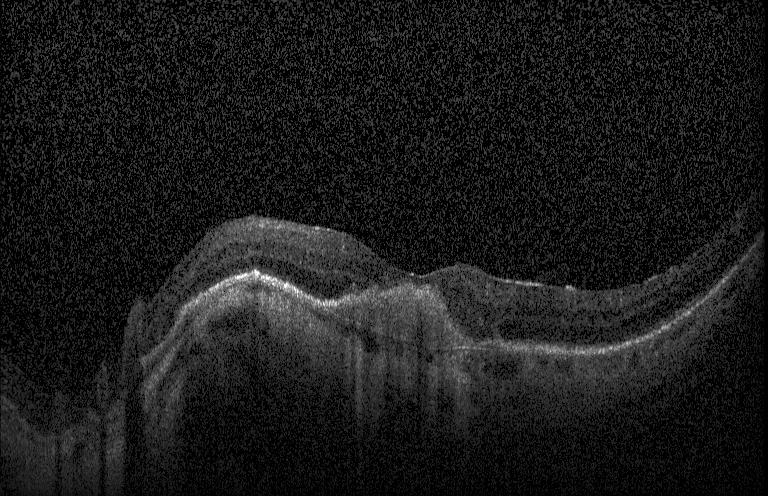

OCT finding: choroidal neovascularization.